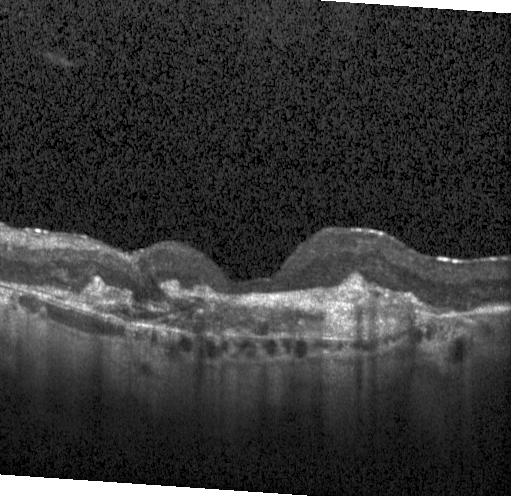 Finding: CNV.